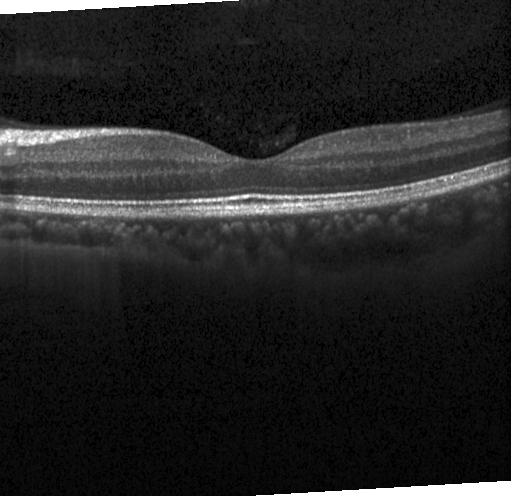
Finding: no choroidal neovascularization, no diabetic macular edema, and no drusen.